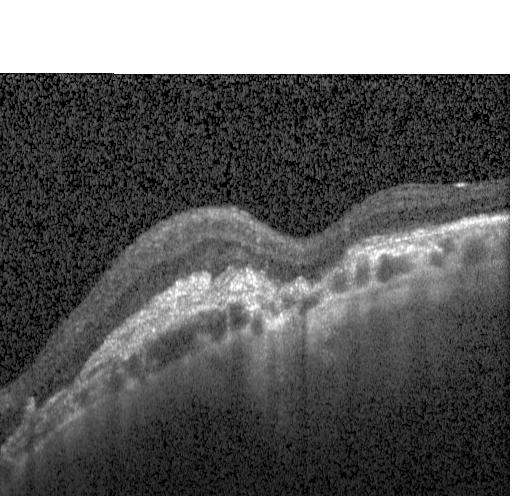
Retinal OCT cross-section — Dx: CNV.